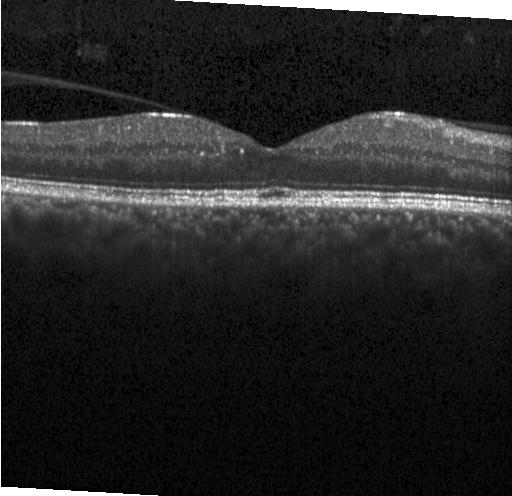

Optical coherence tomography B-scan, spectral-domain optical coherence tomography. OCT finding: neither CNV, DME, nor drusen.